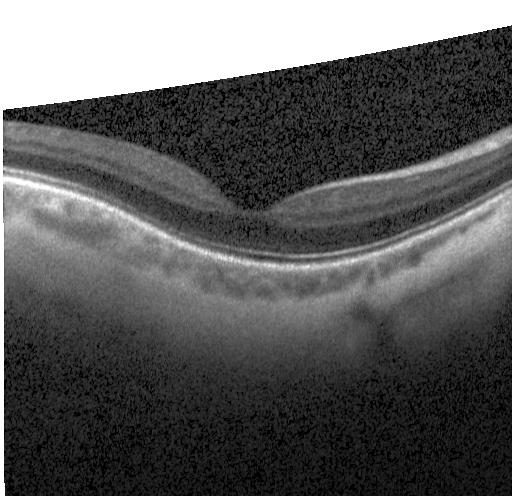 Spectral-domain optical coherence tomography · retinal OCT B-scan · fovea-centered. Finding: no CNV, no DME, and no drusen.